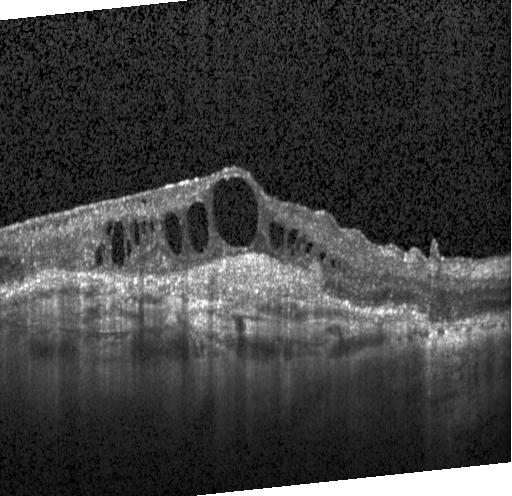
Retinal OCT B-scan. Horizontal scan through the fovea. Spectral-domain optical coherence tomography. Impression: CNV.